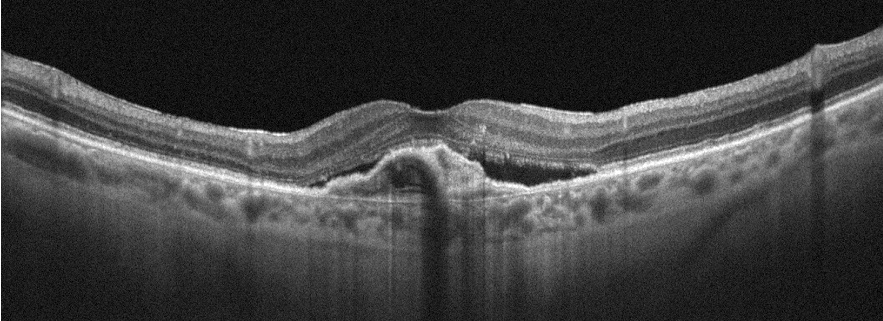 OCT line scan. Through the macula — Assessment: age-related macular degeneration (AMD).